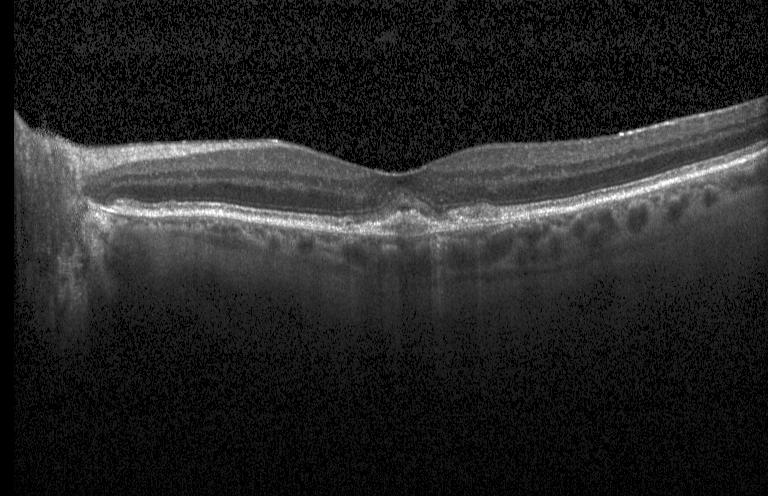

Retinal OCT cross-section showing a choroidal neovascular membrane.